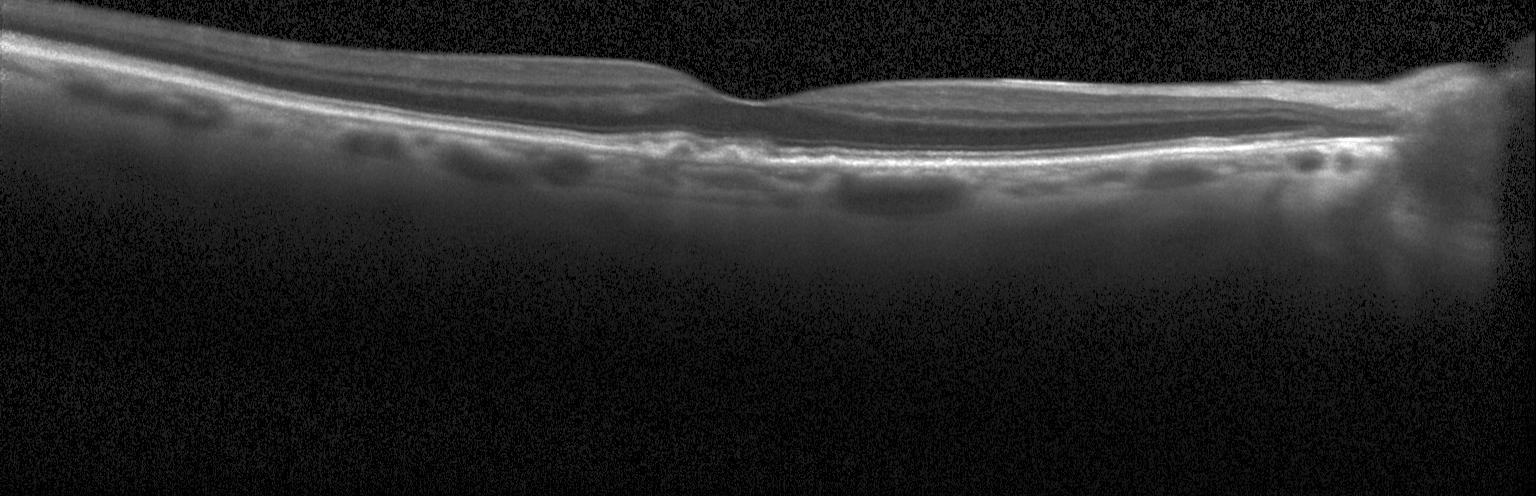

OCT B-scan showing multiple drusen.